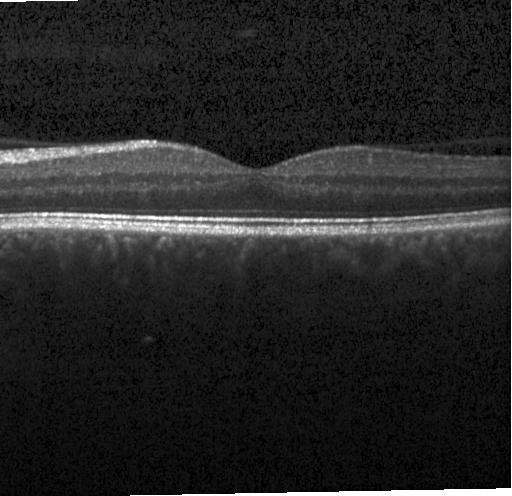 Heidelberg Spectralis OCT system; fovea-centered; optical coherence tomography scan.
OCT finding: no evidence of choroidal neovascularization, diabetic macular edema, or drusen.